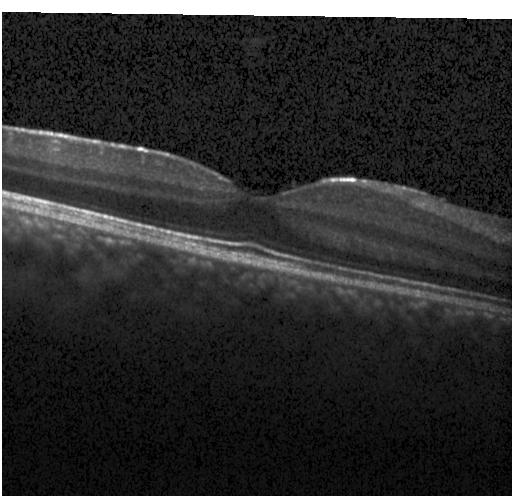
OCT finding: no choroidal neovascularization, no diabetic macular edema, and no drusen.